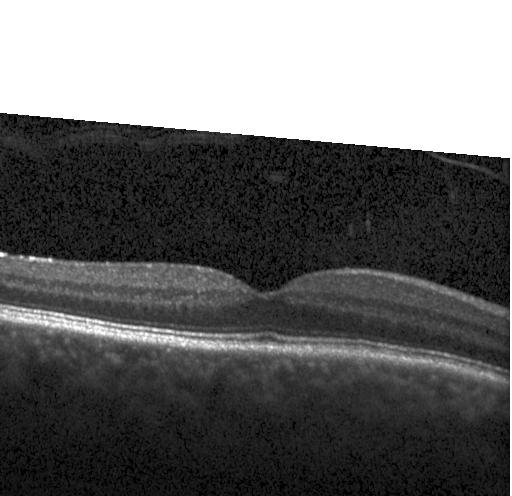
Finding: no choroidal neovascularization, no diabetic macular edema, and no drusen.